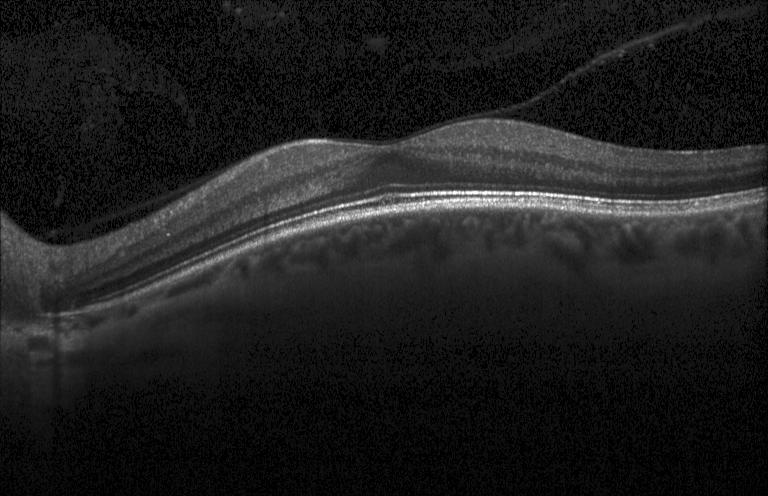

OCT finding: no evidence of choroidal neovascularization, diabetic macular edema, or drusen.